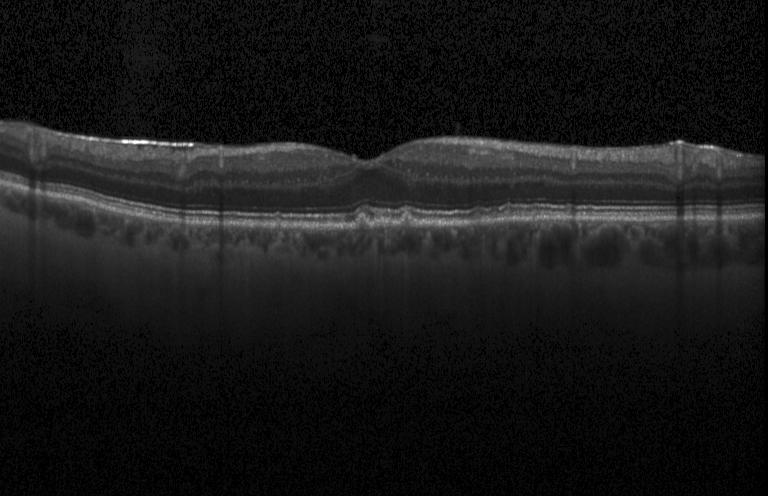
Spectral-domain optical coherence tomography. Heidelberg Spectralis OCT system. Horizontal scan through the fovea. Retinal OCT cross-section.
Dx: drusen.